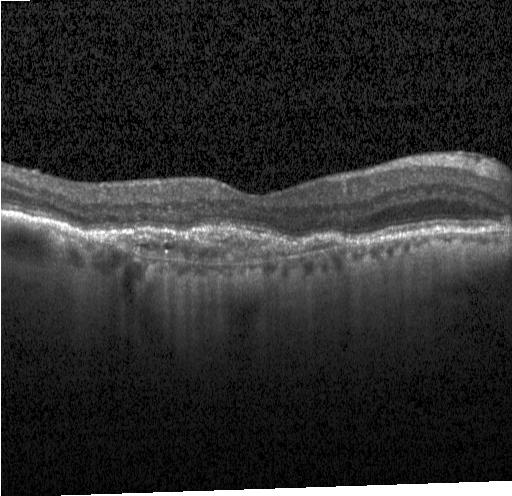
Through the macula · retinal OCT cross-section · instrument: Heidelberg Spectralis · SD-OCT
Diagnosis: a choroidal neovascular membrane.